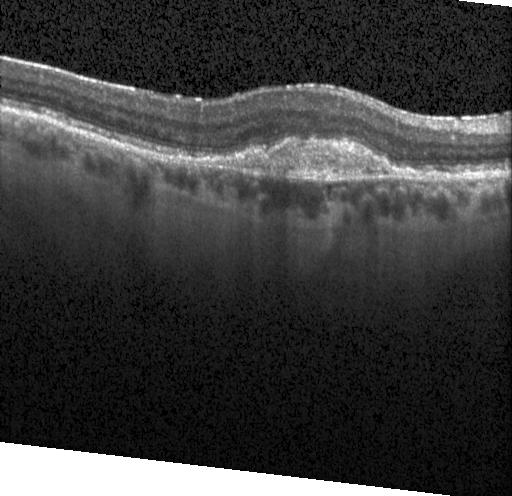 Finding: a choroidal neovascular membrane.